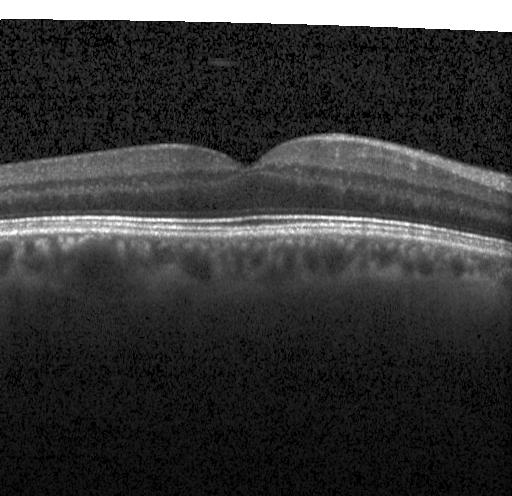

Optical coherence tomography B-scan, spectral-domain OCT, through the macula
Impression: neither CNV, DME, nor drusen.